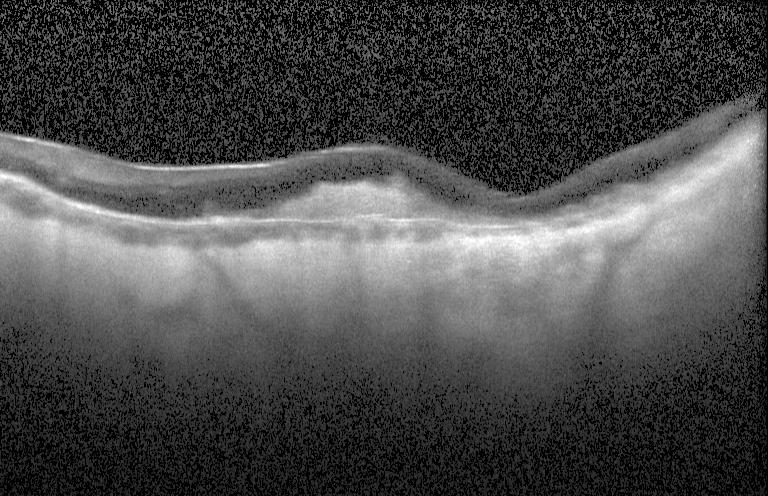
Heidelberg Spectralis OCT system, optical coherence tomography scan, centered on the fovea. Impression: a choroidal neovascular membrane.